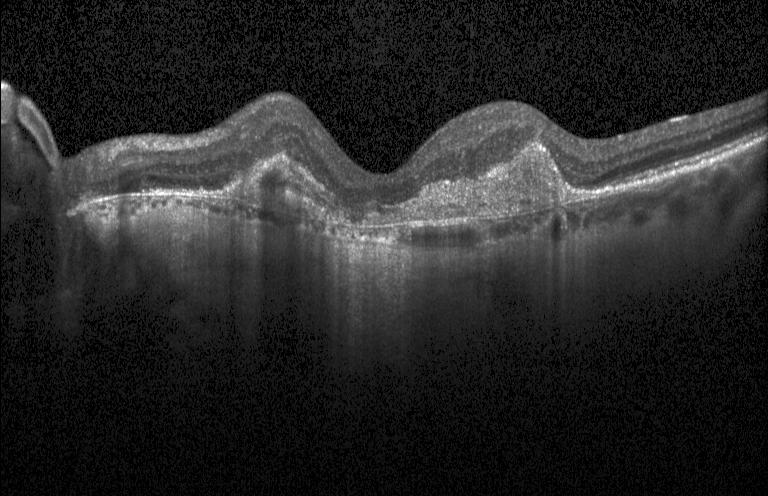

OCT line scan, Heidelberg Spectralis OCT system — Finding: a choroidal neovascular membrane.